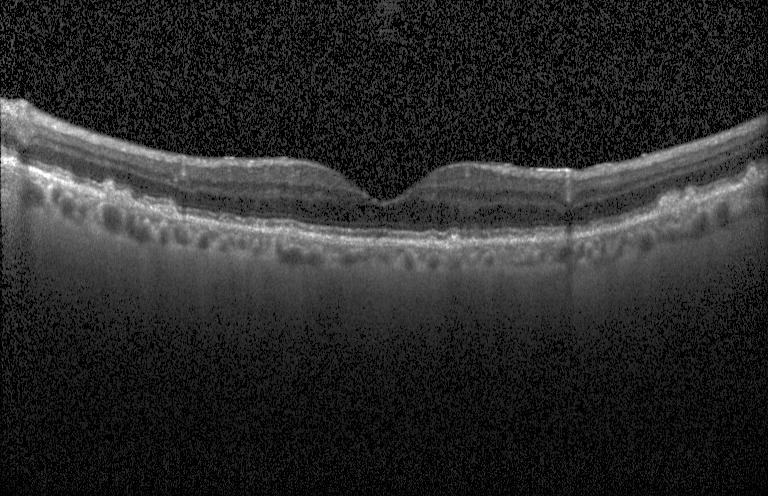
Assessment: multiple drusen.